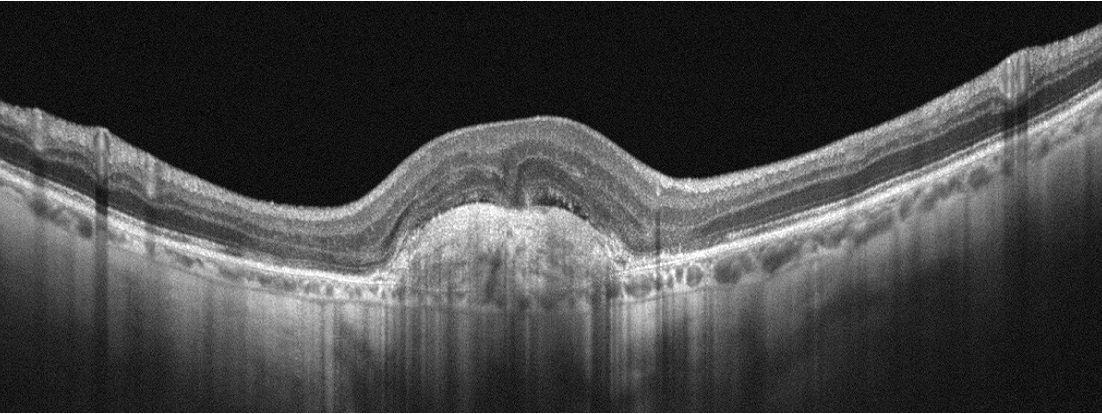 Optical coherence tomography scan.
AMD.